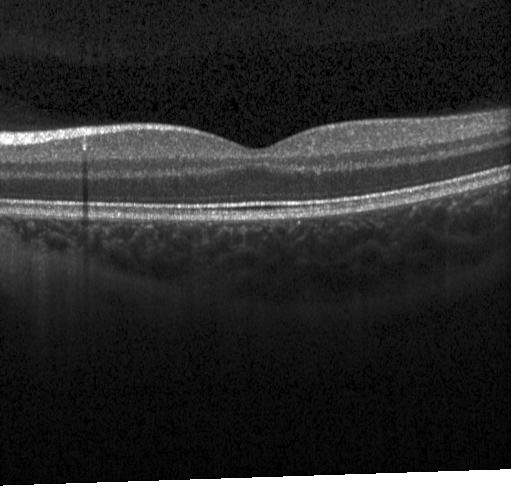
OCT line scan, macular scan
Finding: no CNV, no DME, and no drusen.